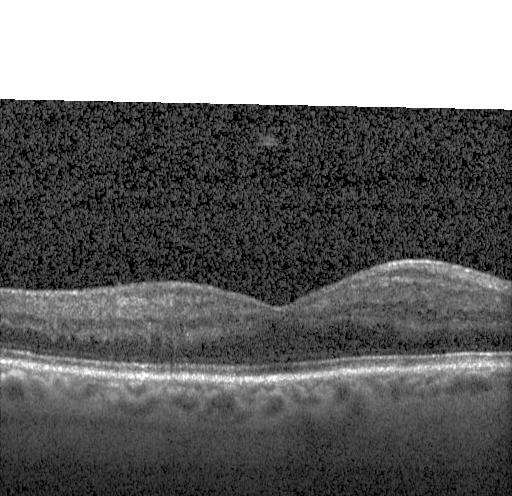
Optical coherence tomography scan.
This B-scan demonstrates neither CNV, DME, nor drusen.